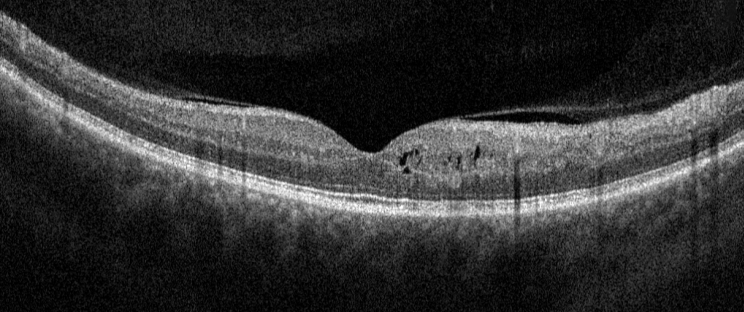
OCT line scan; through the macula. Assessment: diabetic macular edema.